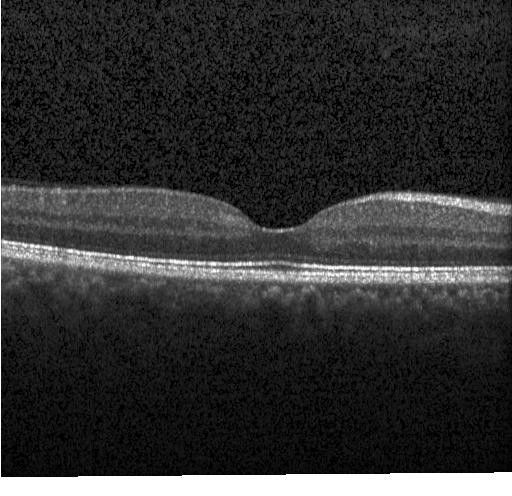 OCT line scan — OCT finding: no choroidal neovascularization, diabetic macular edema, or drusen.